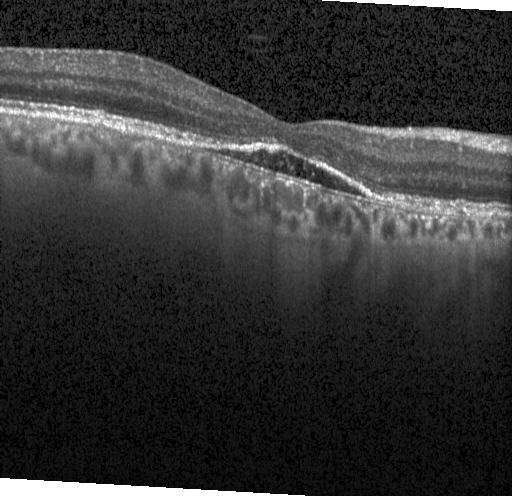 Optical coherence tomography B-scan, SD-OCT, acquired on a Heidelberg Spectralis
Finding: a choroidal neovascular membrane.